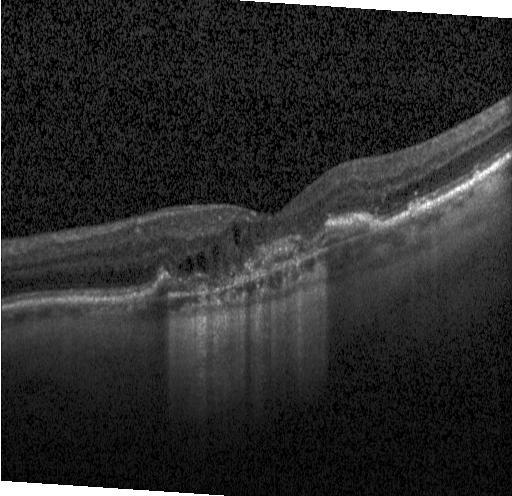

Diagnosis: a choroidal neovascular membrane.